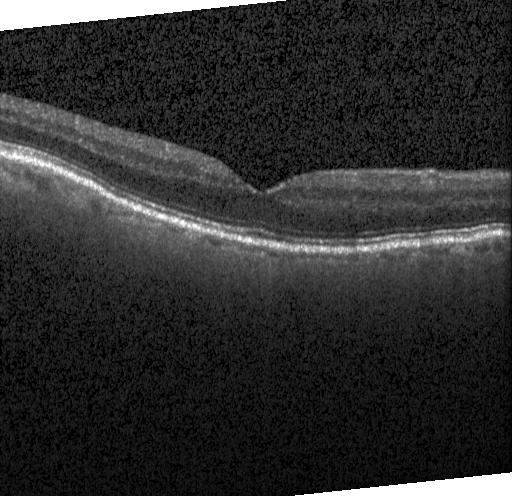 Optical coherence tomography B-scan. The scan shows neither choroidal neovascularization, diabetic macular edema, nor drusen.